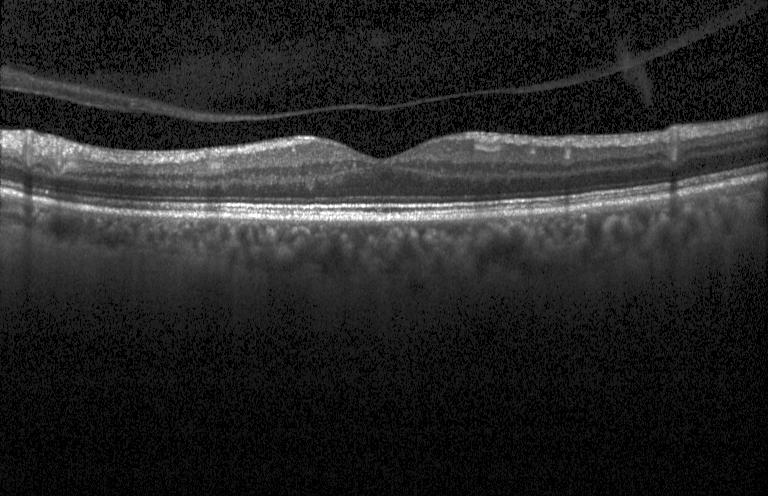
Assessment: no choroidal neovascularization, diabetic macular edema, or drusen.